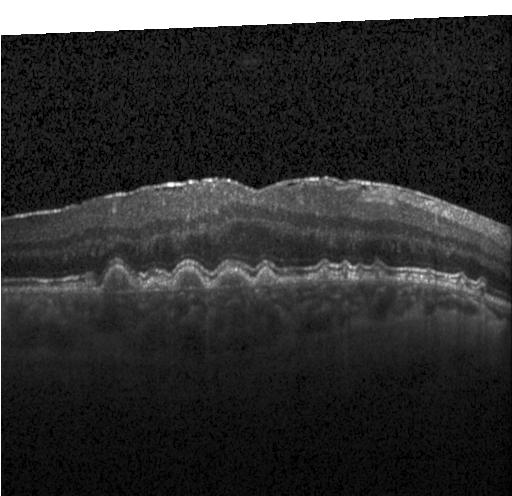

Fovea-centered; optical coherence tomography B-scan — The scan shows drusen.